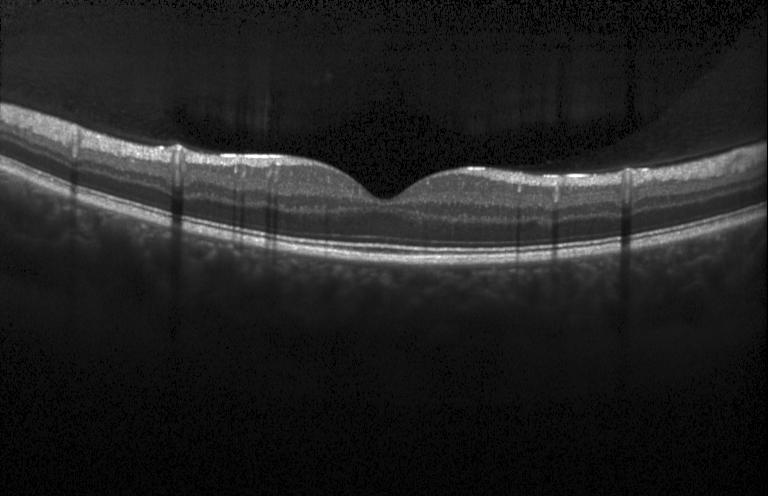
SD-OCT · OCT B-scan.
The scan shows no choroidal neovascularization, diabetic macular edema, or drusen.